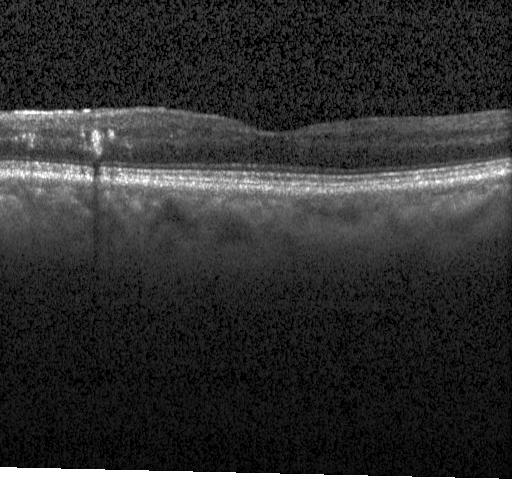
Heidelberg Spectralis OCT system. Horizontal scan through the fovea. Spectral-domain optical coherence tomography. Retinal OCT cross-section
Assessment: no choroidal neovascularization, no diabetic macular edema, and no drusen.